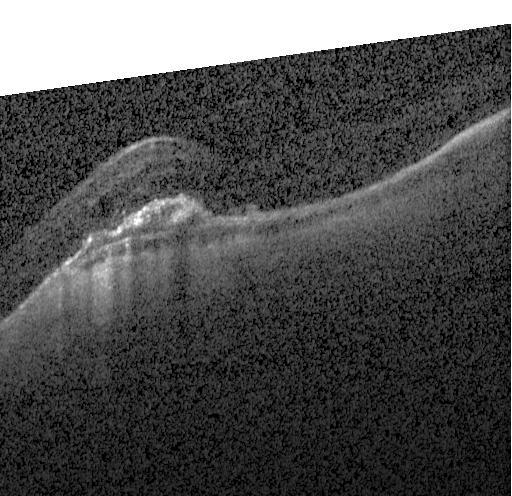
OCT scan showing a choroidal neovascular membrane.